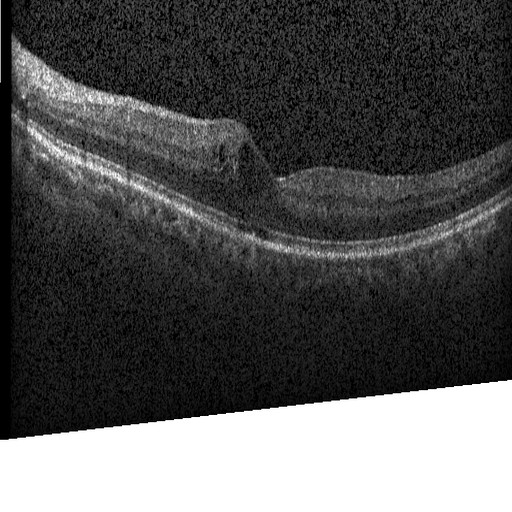

Impression: diabetic macular edema (DME).